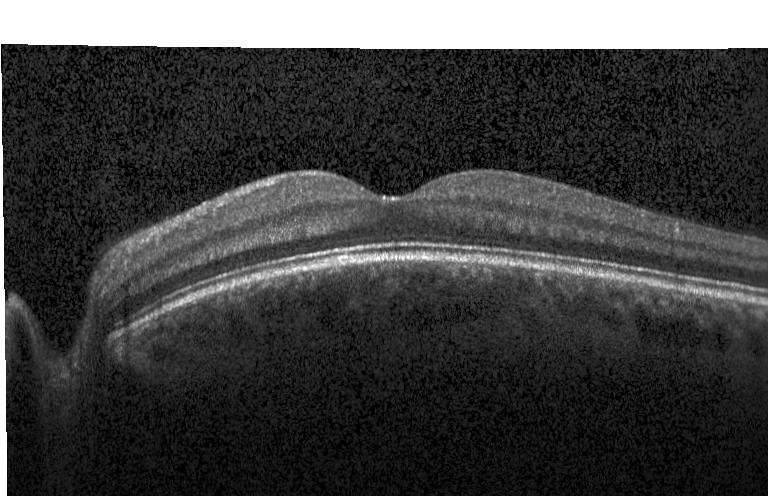

OCT scan showing neither choroidal neovascularization, diabetic macular edema, nor drusen.